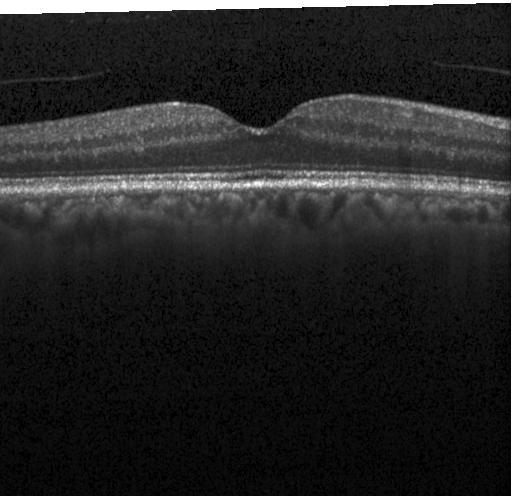 OCT finding: no evidence of choroidal neovascularization, diabetic macular edema, or drusen.